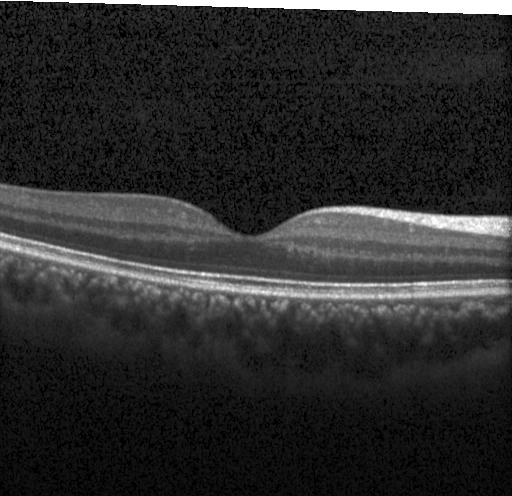
Assessment: no CNV, DME, or drusen.